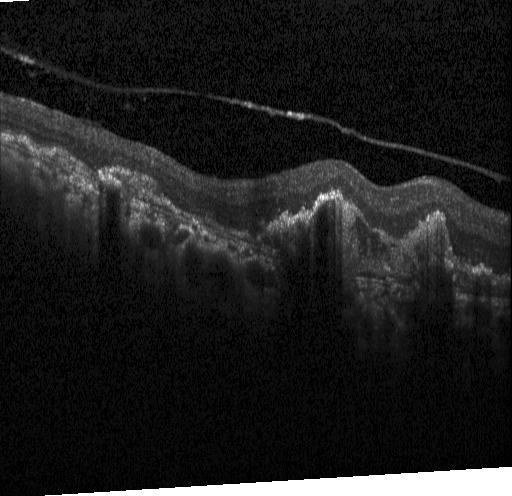

Impression: choroidal neovascularization (CNV).